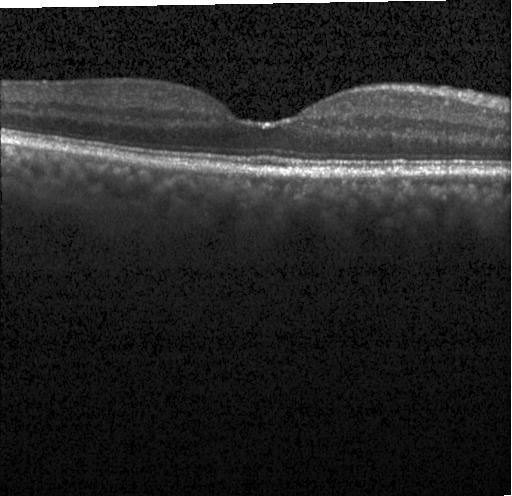

This B-scan demonstrates no choroidal neovascularization, diabetic macular edema, or drusen.